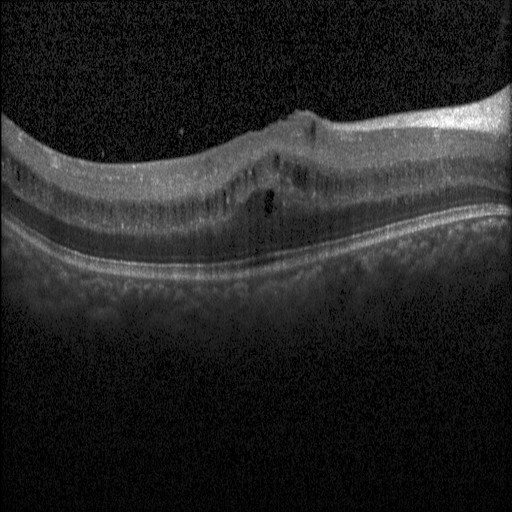 Dx: diabetic macular edema.